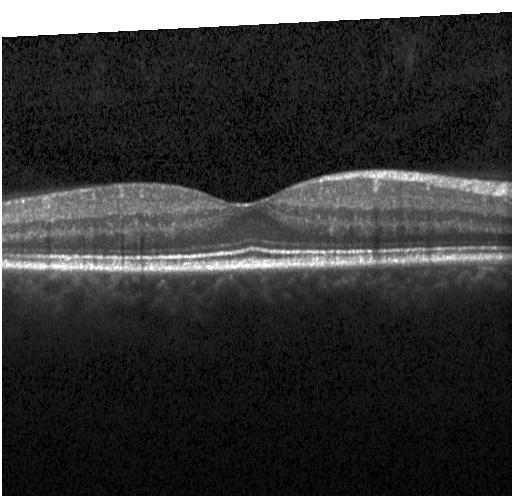 Optical coherence tomography B-scan
OCT finding: no choroidal neovascularization, diabetic macular edema, or drusen.